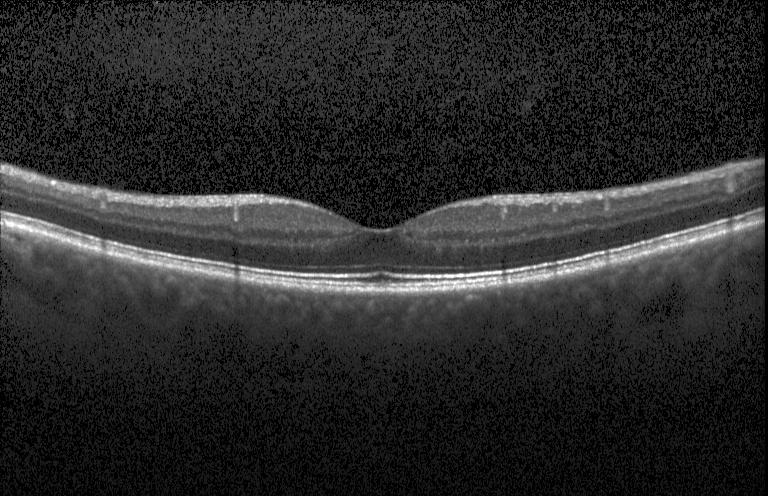 Finding: neither CNV, DME, nor drusen.